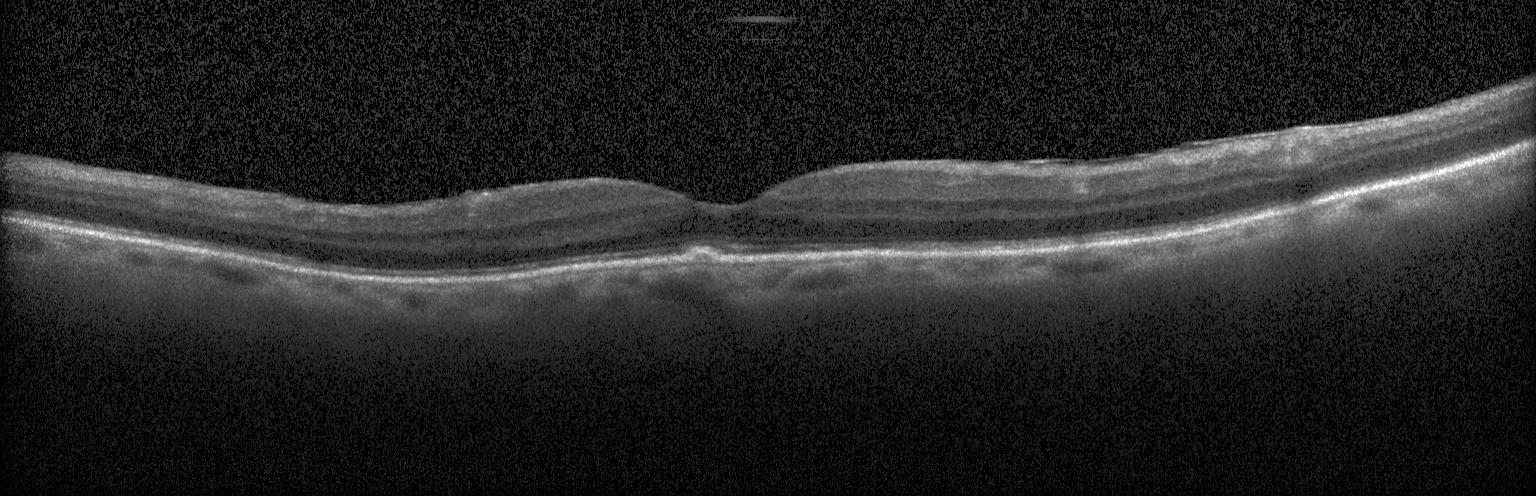
Macular scan. Instrument: Heidelberg Spectralis. OCT line scan. SD-OCT
Diagnosis: sub-RPE drusenoid deposits.